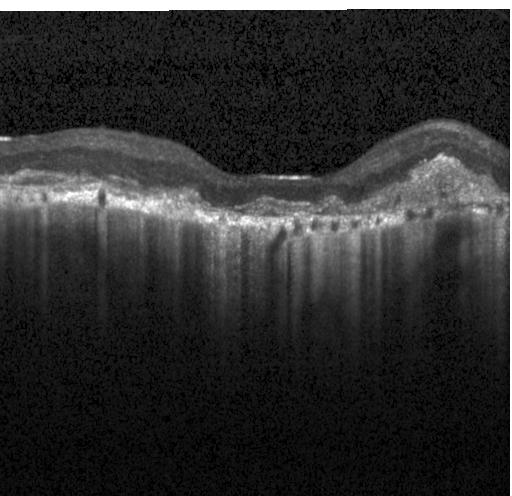
Acquired on a Heidelberg Spectralis · fovea-centered · OCT line scan · spectral-domain optical coherence tomography — Choroidal neovascularization (CNV).